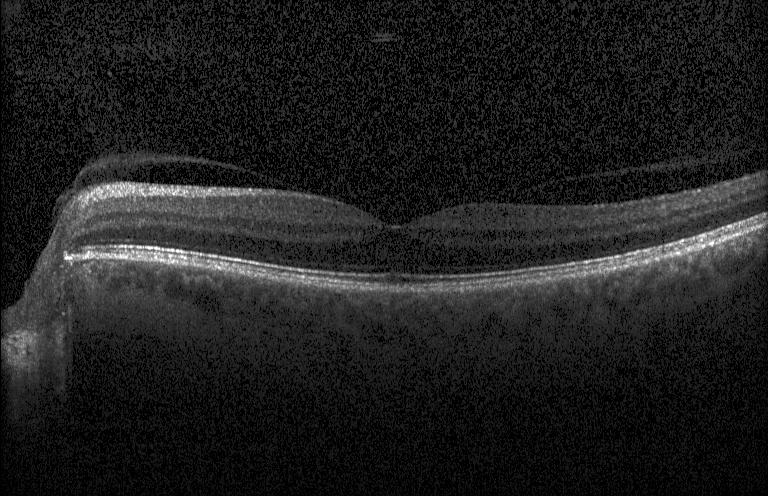

Spectral-domain OCT. Fovea-centered. Heidelberg Spectralis. Retinal OCT cross-section — No choroidal neovascularization, diabetic macular edema, or drusen.